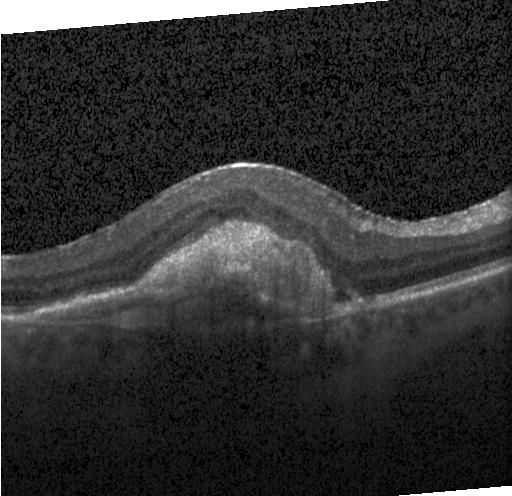
OCT line scan. OCT finding: a choroidal neovascular membrane.